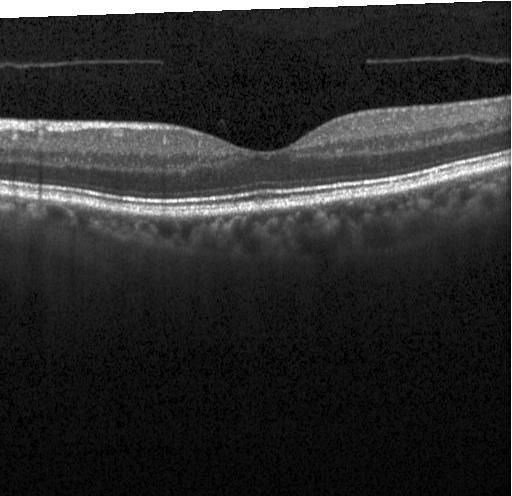
Retinal OCT cross-section. Macular scan. Spectral-domain OCT.
This B-scan demonstrates no choroidal neovascularization, no diabetic macular edema, and no drusen.